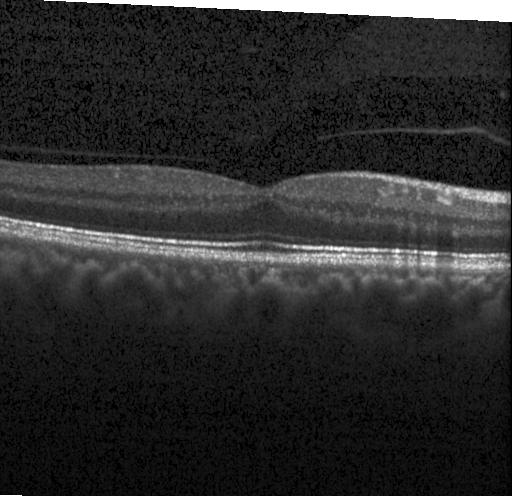 Acquired on a Heidelberg Spectralis, spectral-domain OCT, OCT B-scan, horizontal scan through the fovea. Impression: neither choroidal neovascularization, diabetic macular edema, nor drusen.